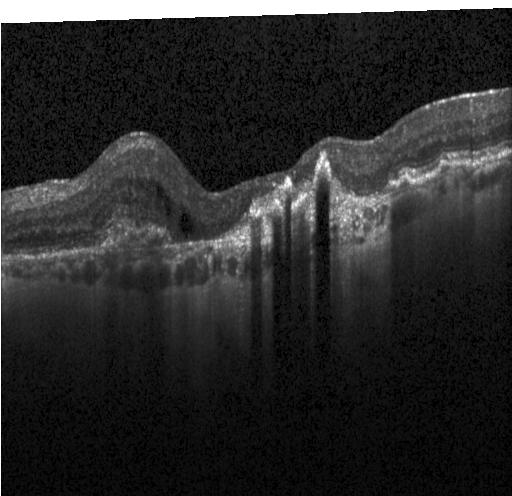 Retinal OCT cross-section; through the macula; instrument: Heidelberg Spectralis; spectral-domain optical coherence tomography — Assessment: CNV.